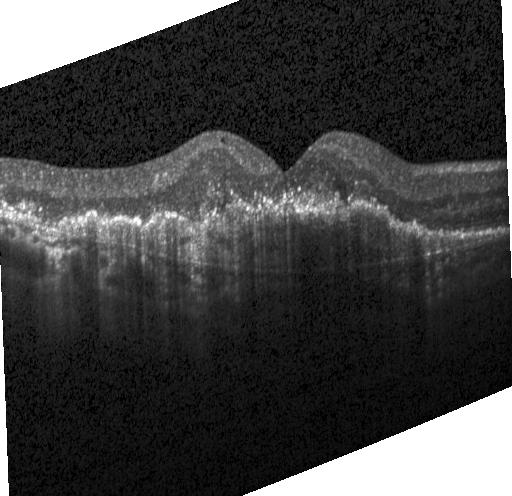
Assessment: choroidal neovascularization.